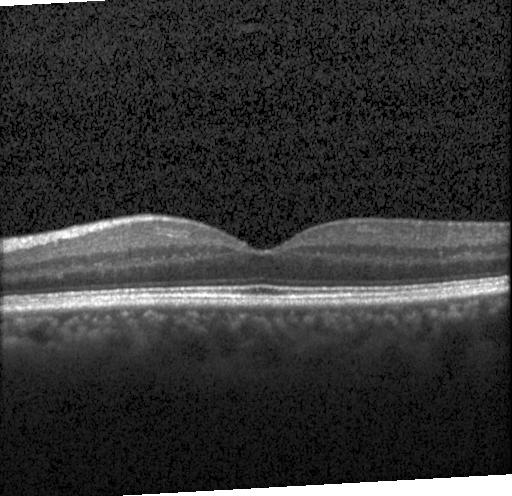 Retinal OCT B-scan. Diagnosis: no evidence of CNV, DME, or drusen.